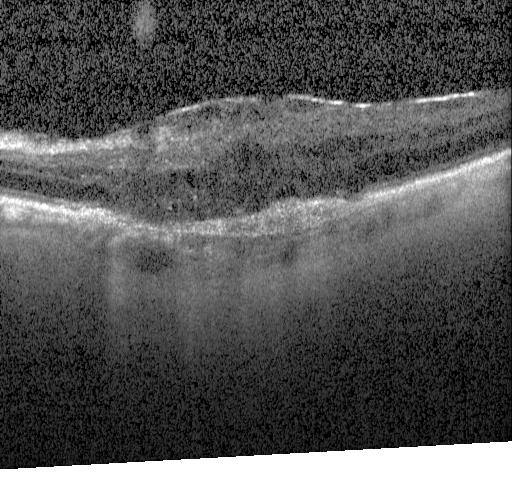
OCT scan showing a choroidal neovascular membrane.